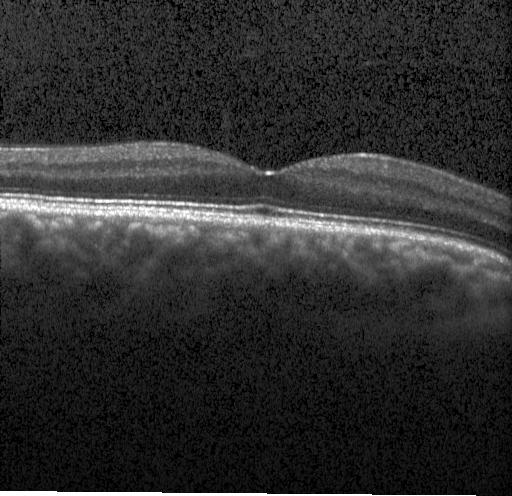

OCT B-scan showing neither CNV, DME, nor drusen.